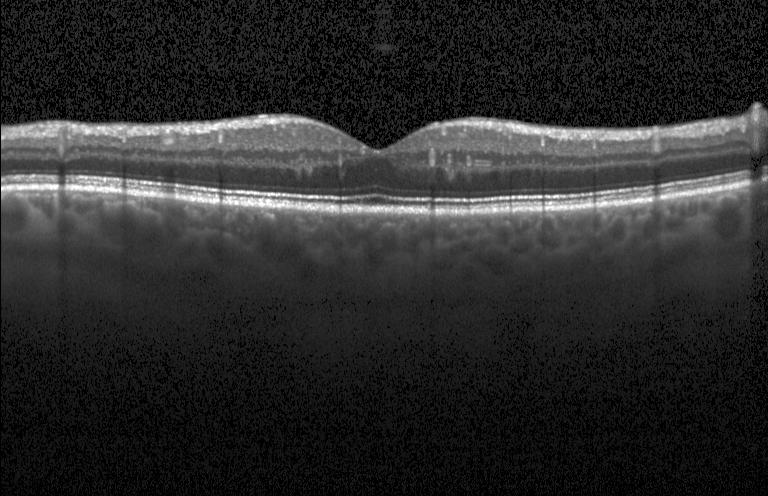 Optical coherence tomography B-scan, SD-OCT, instrument: Heidelberg Spectralis.
Finding: no choroidal neovascularization, diabetic macular edema, or drusen.